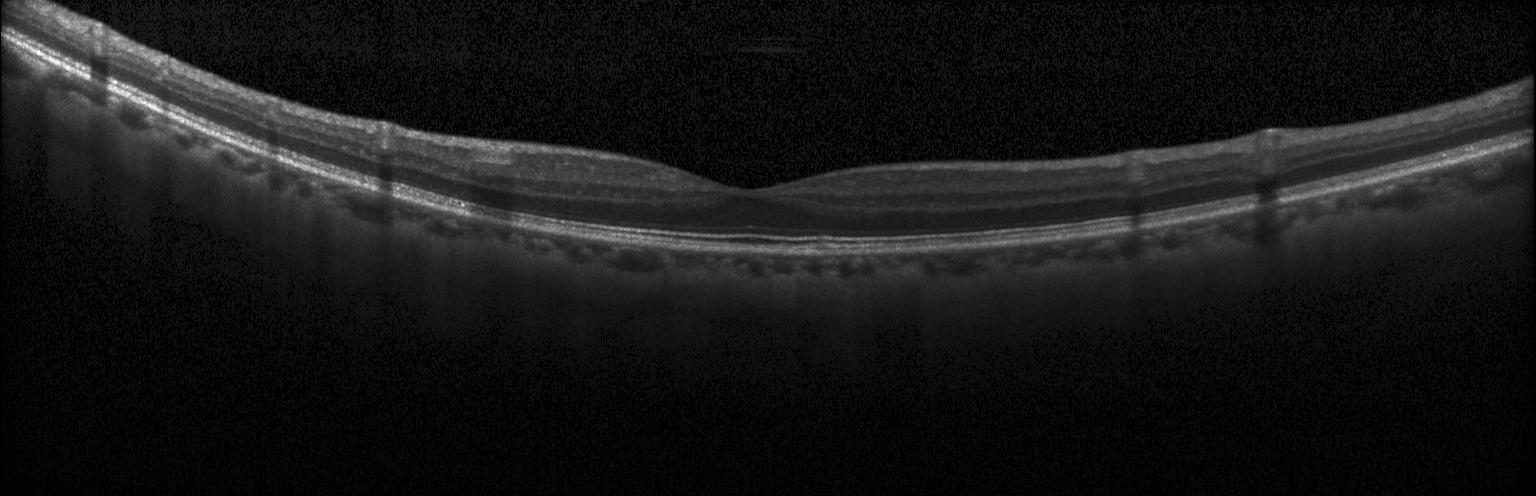 OCT B-scan — This B-scan demonstrates no choroidal neovascularization, no diabetic macular edema, and no drusen.